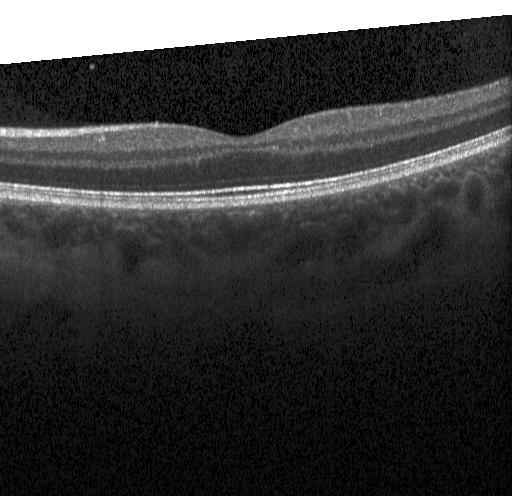 Horizontal scan through the fovea; optical coherence tomography B-scan; spectral-domain OCT
Diagnosis: no choroidal neovascularization, diabetic macular edema, or drusen.